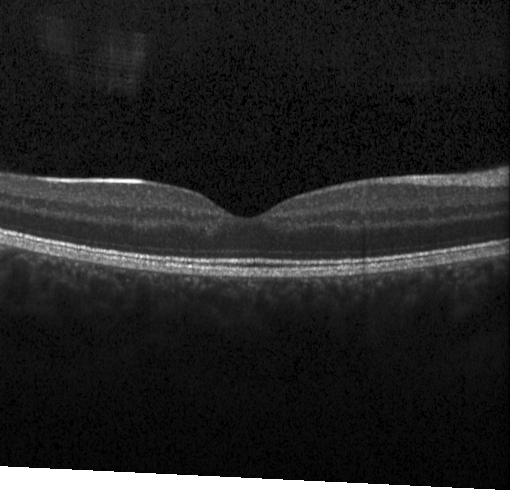

Impression: no choroidal neovascularization, diabetic macular edema, or drusen.